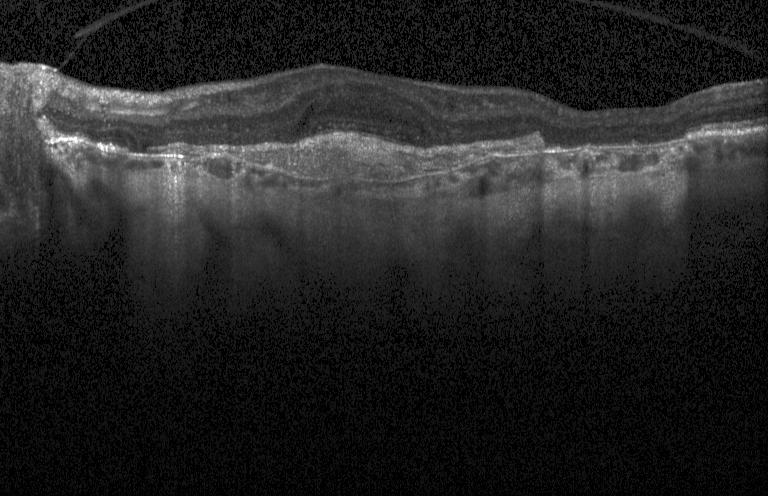 Diagnosis: a choroidal neovascular membrane.